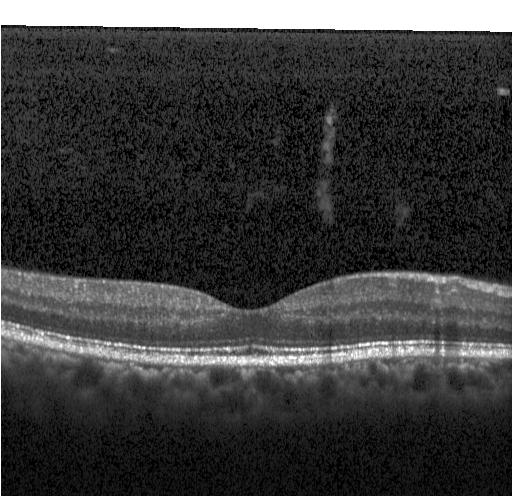
Optical coherence tomography scan. No choroidal neovascularization, diabetic macular edema, or drusen.